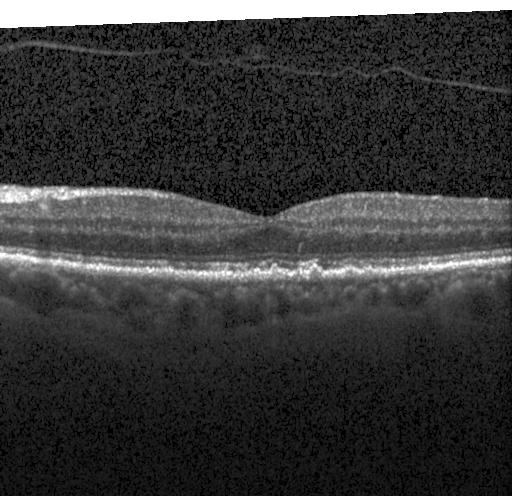
Optical coherence tomography B-scan, acquired on a Heidelberg Spectralis, spectral-domain OCT, horizontal scan through the fovea
Multiple drusen.